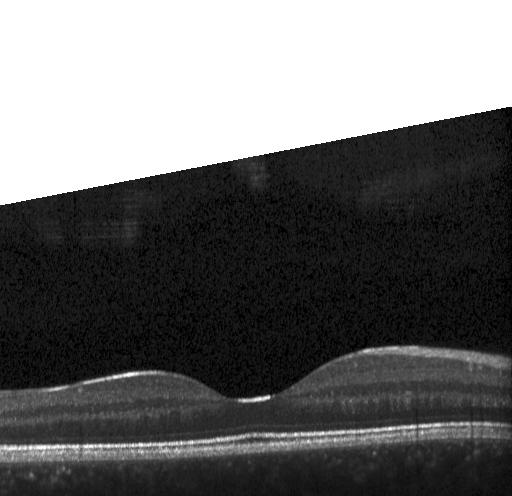
OCT finding: neither CNV, DME, nor drusen.